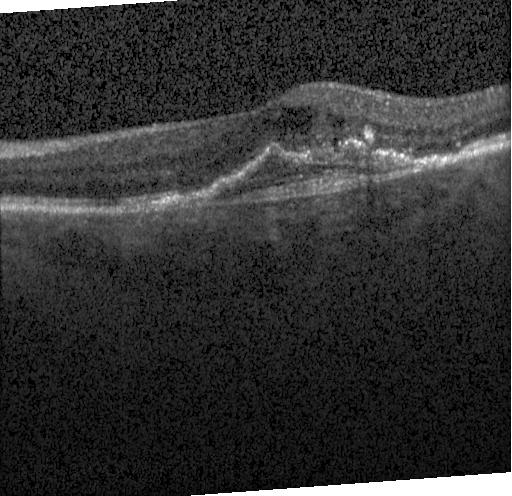 OCT scan showing choroidal neovascularization.